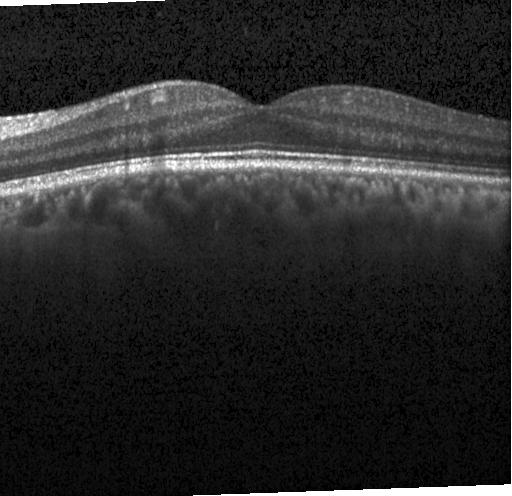

OCT B-scan showing no choroidal neovascularization, diabetic macular edema, or drusen.